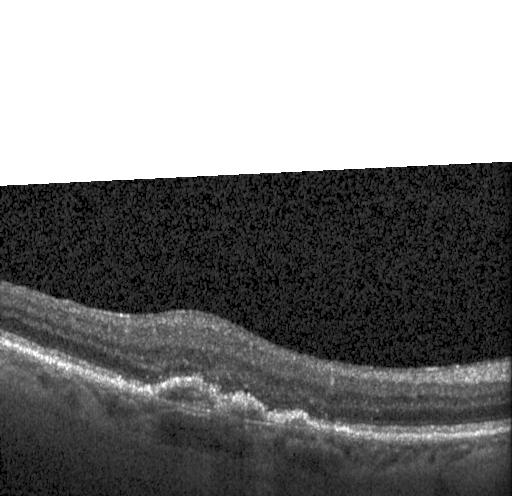

The scan shows choroidal neovascularization.